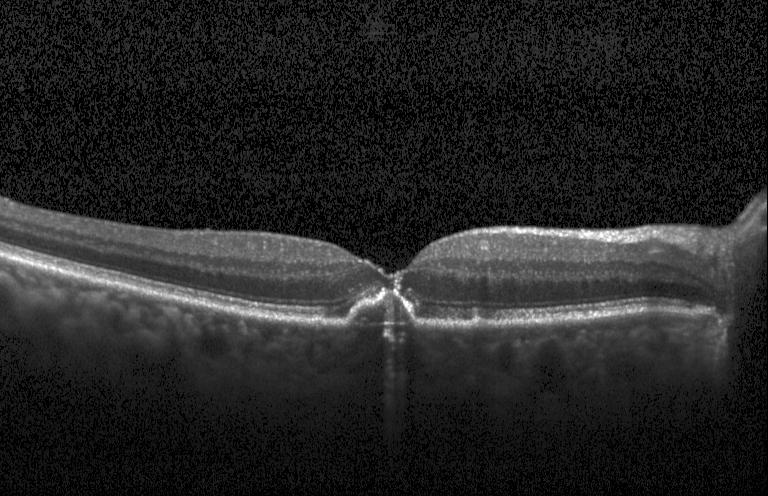 Diagnosis: choroidal neovascularization.